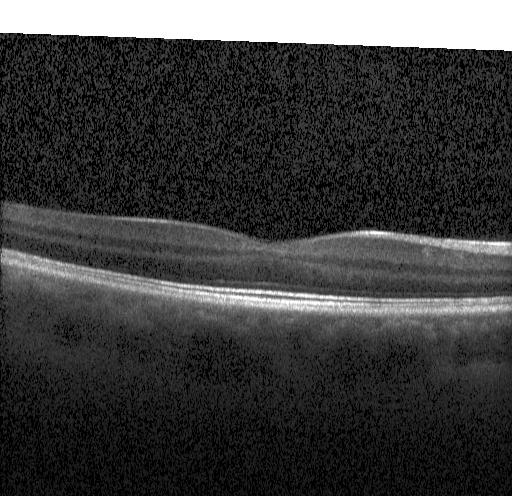

OCT line scan, Heidelberg Spectralis — Assessment: no choroidal neovascularization, no diabetic macular edema, and no drusen.